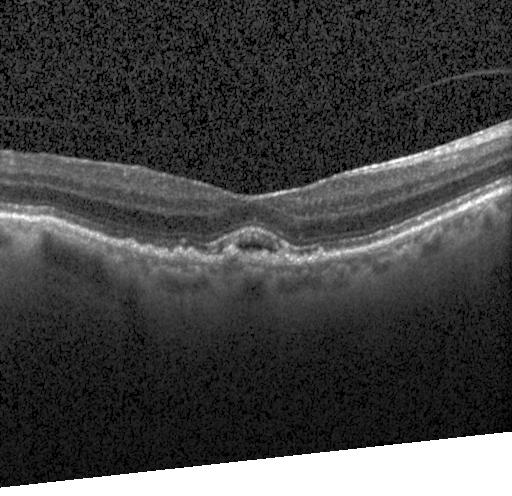
SD-OCT. Optical coherence tomography scan. Centered on the fovea.
Finding: choroidal neovascularization.